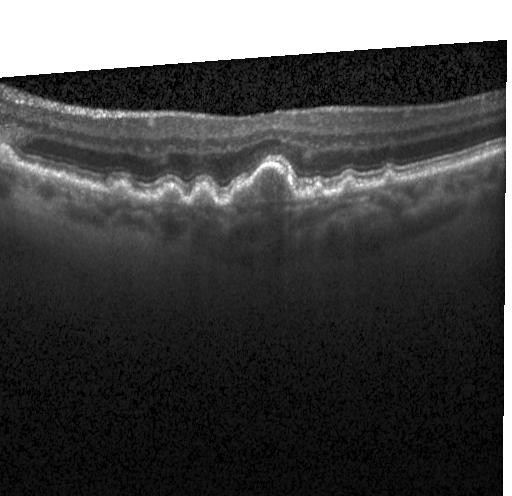
OCT scan showing multiple drusen.